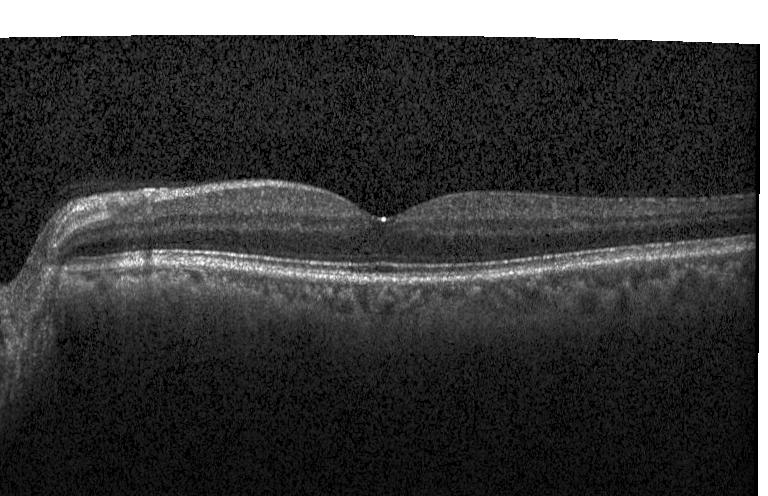 Retinal OCT cross-section · acquired on a Heidelberg Spectralis · through the macula — Impression: neither CNV, DME, nor drusen.